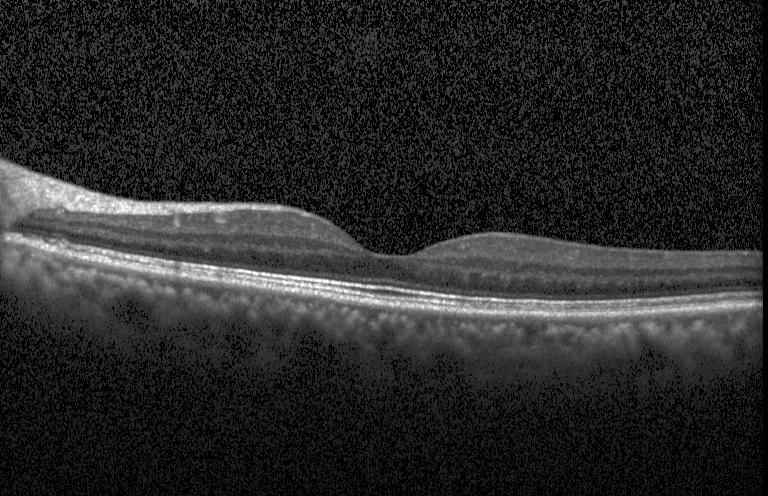
Retinal OCT cross-section. Heidelberg Spectralis. SD-OCT.
OCT finding: neither CNV, DME, nor drusen.